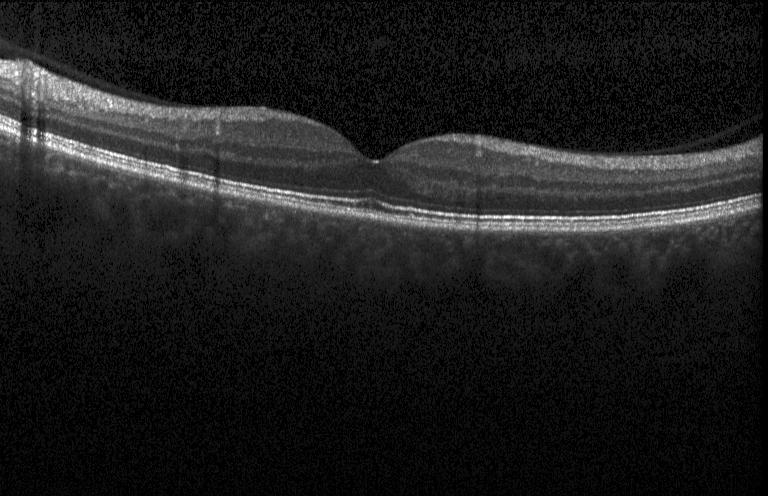
OCT line scan
OCT finding: no choroidal neovascularization, no diabetic macular edema, and no drusen.